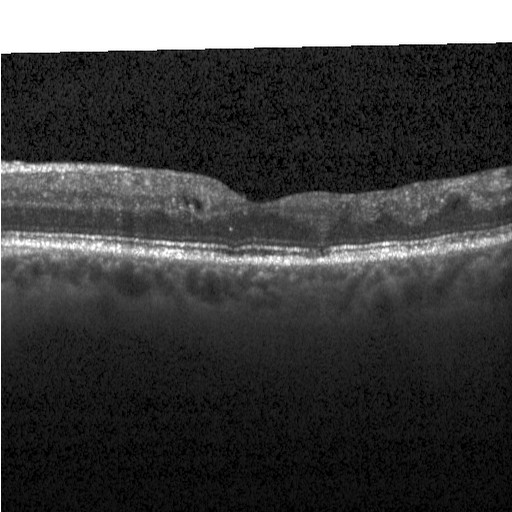 Optical coherence tomography B-scan · spectral-domain OCT.
Impression: diabetic macular edema (DME).